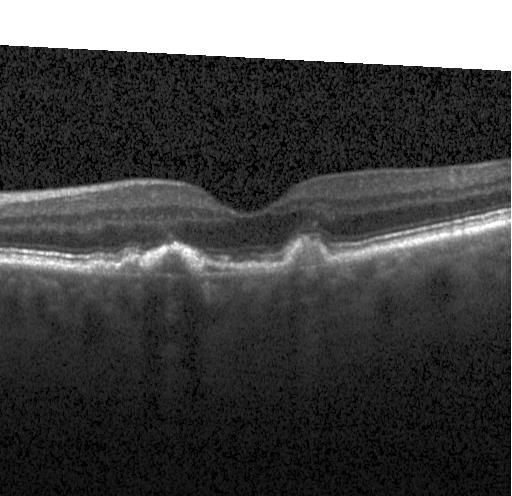 Retinal OCT cross-section. Diagnosis: choroidal neovascularization.